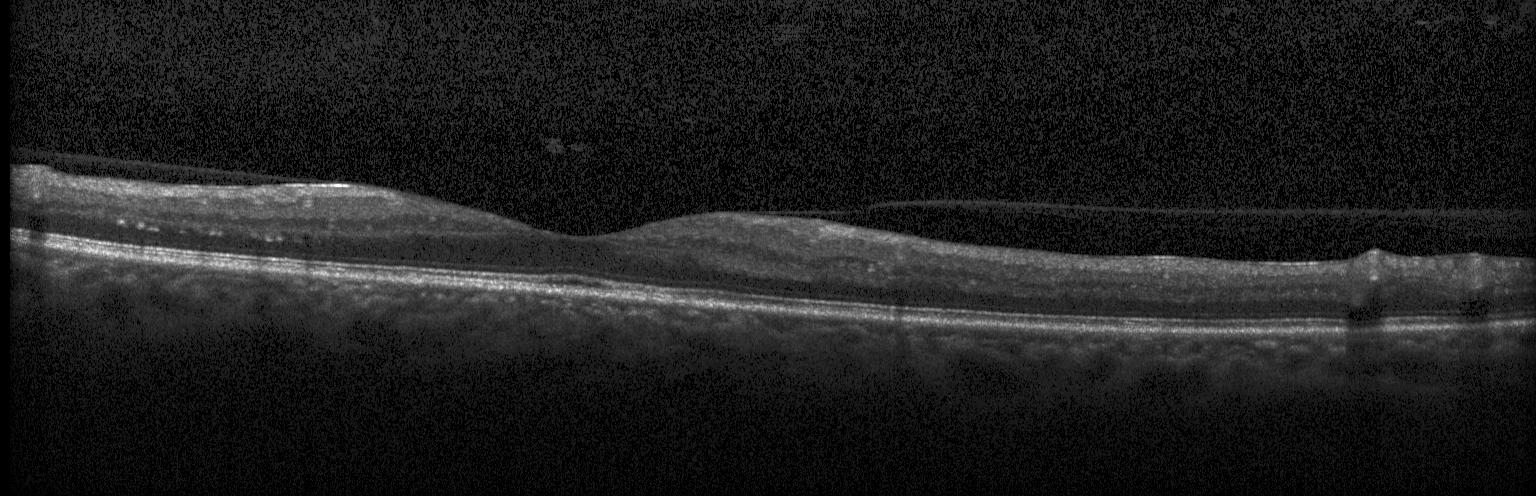 OCT line scan · spectral-domain optical coherence tomography.
Diagnosis: no choroidal neovascularization, diabetic macular edema, or drusen.